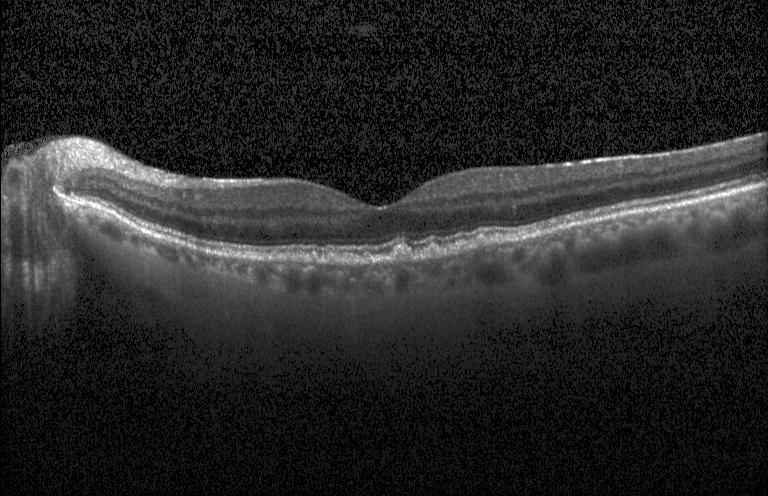 Optical coherence tomography scan.
Diagnosis: drusen.